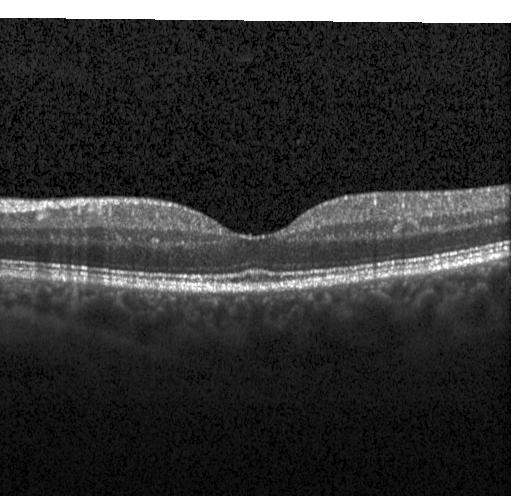

Spectral-domain OCT, through the macula, acquired on a Heidelberg Spectralis, optical coherence tomography scan
No CNV, DME, or drusen.